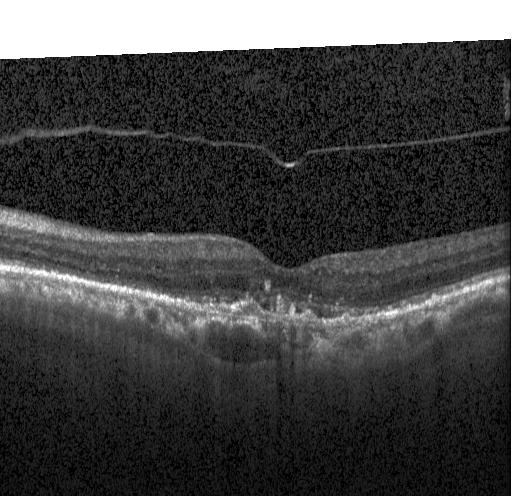
Spectral-domain OCT B-scan: choroidal neovascularization (CNV).